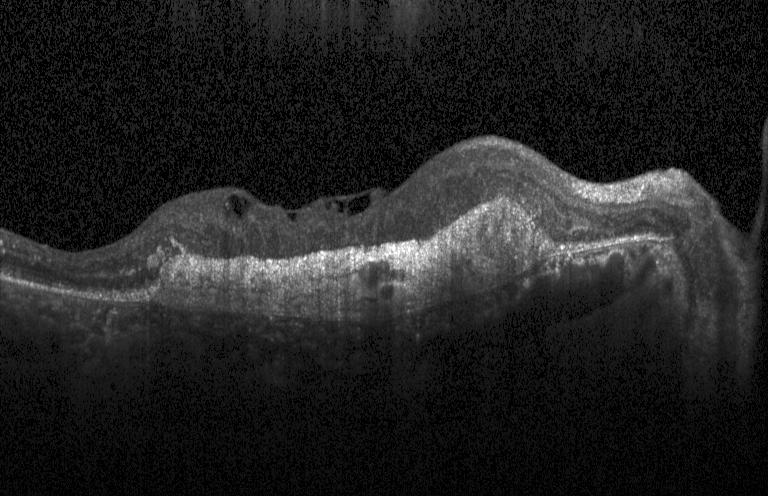
A choroidal neovascular membrane.